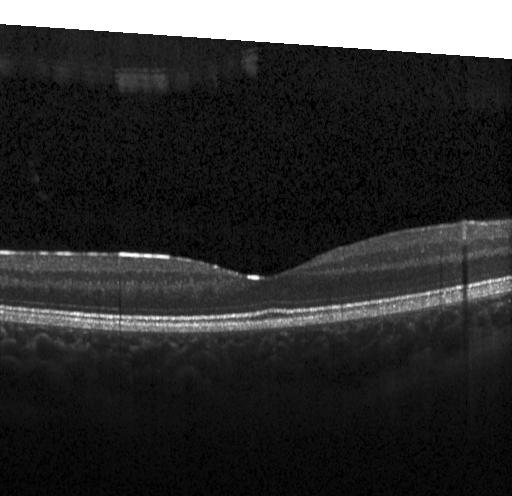 Diagnosis: no choroidal neovascularization, no diabetic macular edema, and no drusen.